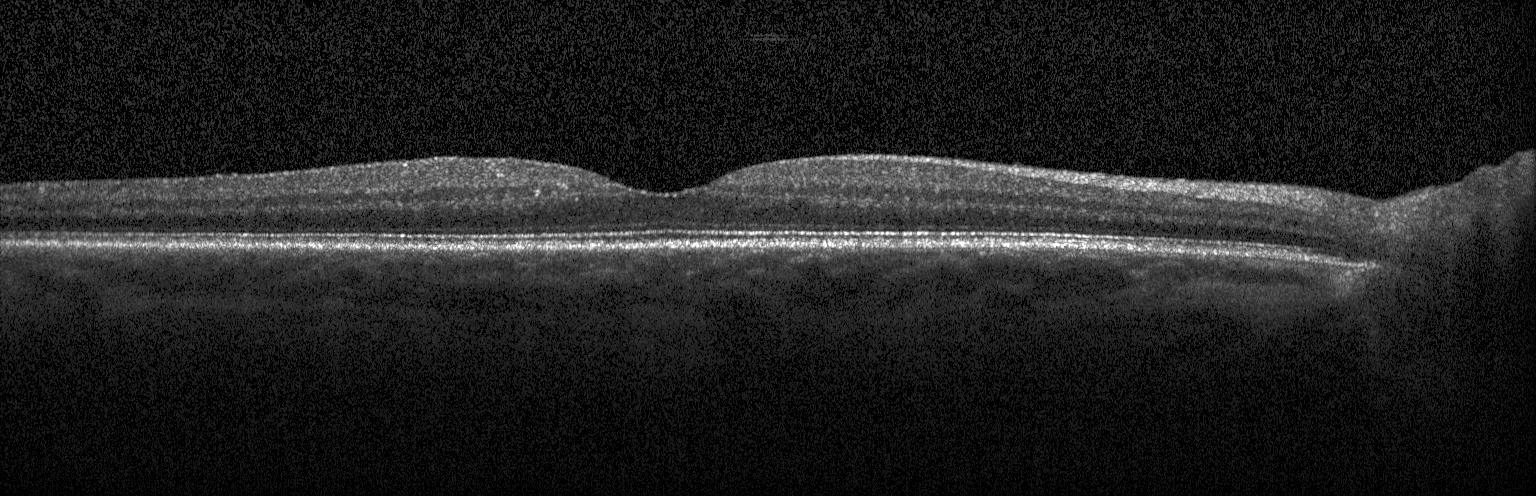

Finding: no CNV, no DME, and no drusen.